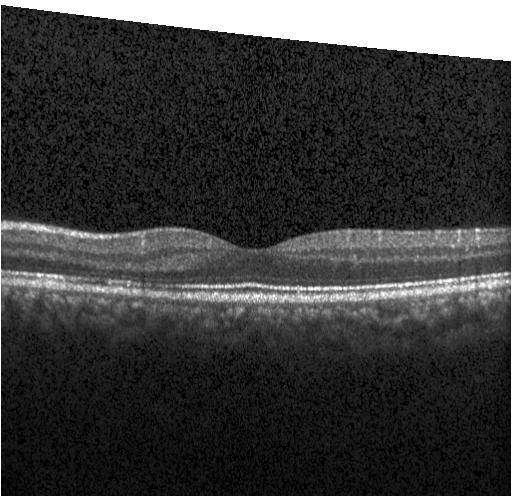
Optical coherence tomography scan
Impression: no CNV, DME, or drusen.